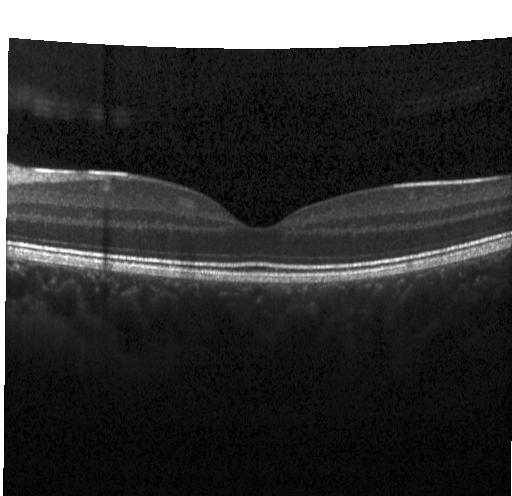 Finding: no evidence of choroidal neovascularization, diabetic macular edema, or drusen.